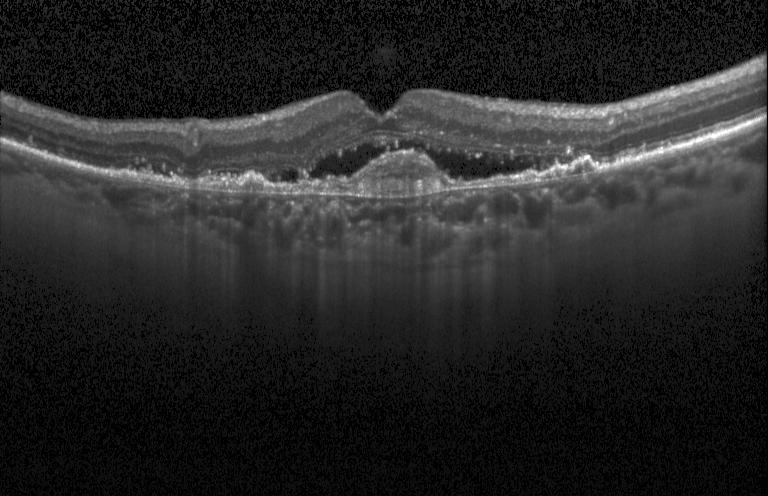 Spectral-domain OCT, Heidelberg Spectralis OCT system, retinal OCT cross-section
Finding: a choroidal neovascular membrane.